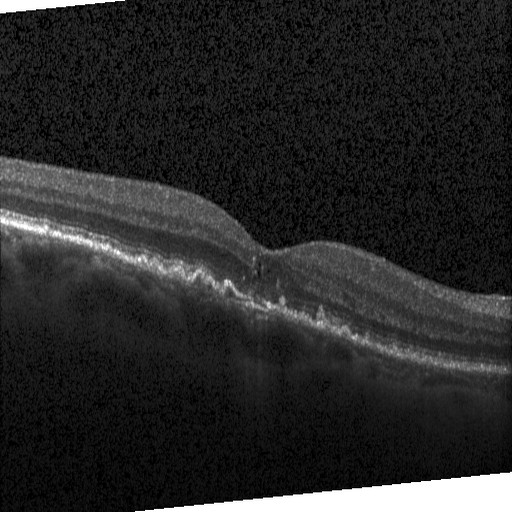

Through the macula, acquired on a Heidelberg Spectralis, retinal OCT B-scan.
Macular OCT: diabetic macular edema.